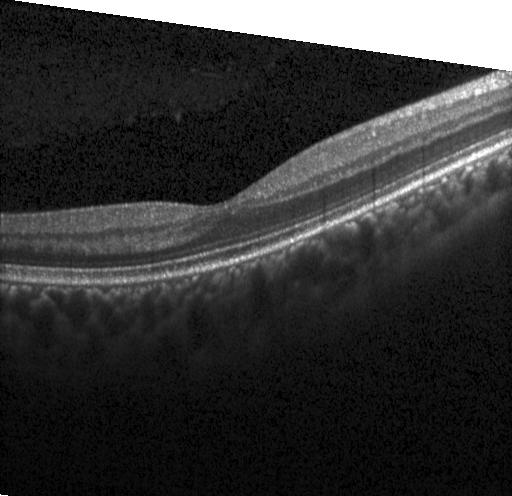

Optical coherence tomography B-scan, fovea-centered. Diagnosis: no choroidal neovascularization, no diabetic macular edema, and no drusen.